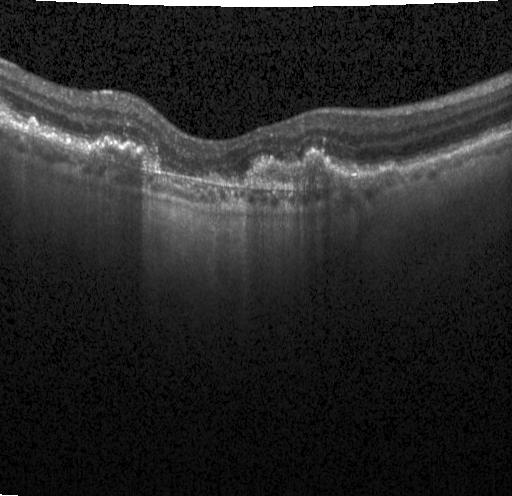
Heidelberg Spectralis. Through the macula. Optical coherence tomography B-scan. SD-OCT.
Finding: a choroidal neovascular membrane.